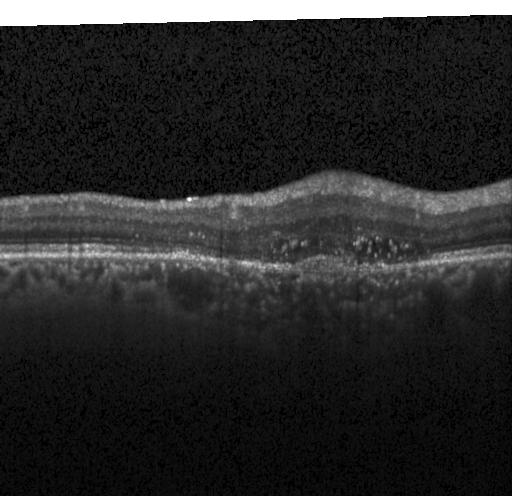
Assessment: a choroidal neovascular membrane.